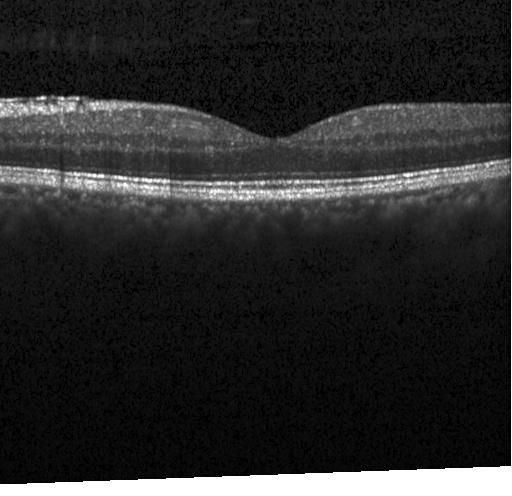 Spectral-domain OCT, fovea-centered, Heidelberg Spectralis OCT system, OCT line scan — This B-scan demonstrates no evidence of CNV, DME, or drusen.